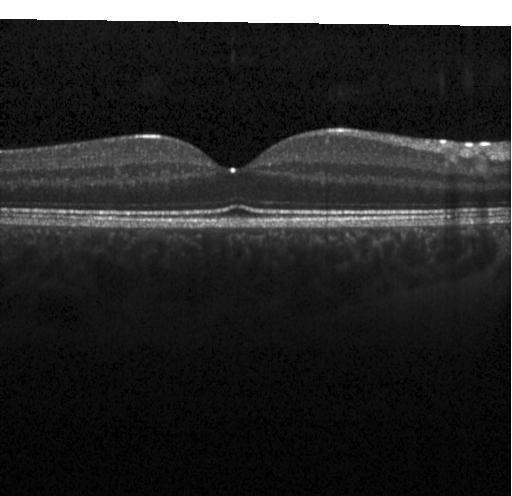 SD-OCT. OCT line scan. Heidelberg Spectralis.
Dx: no evidence of CNV, DME, or drusen.